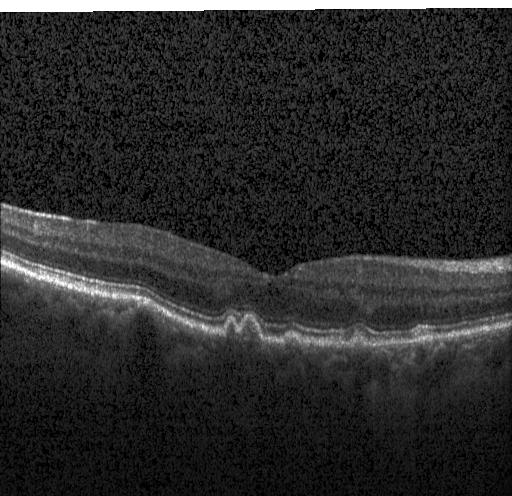 Retinal OCT cross-section; spectral-domain optical coherence tomography
Dx: drusen.